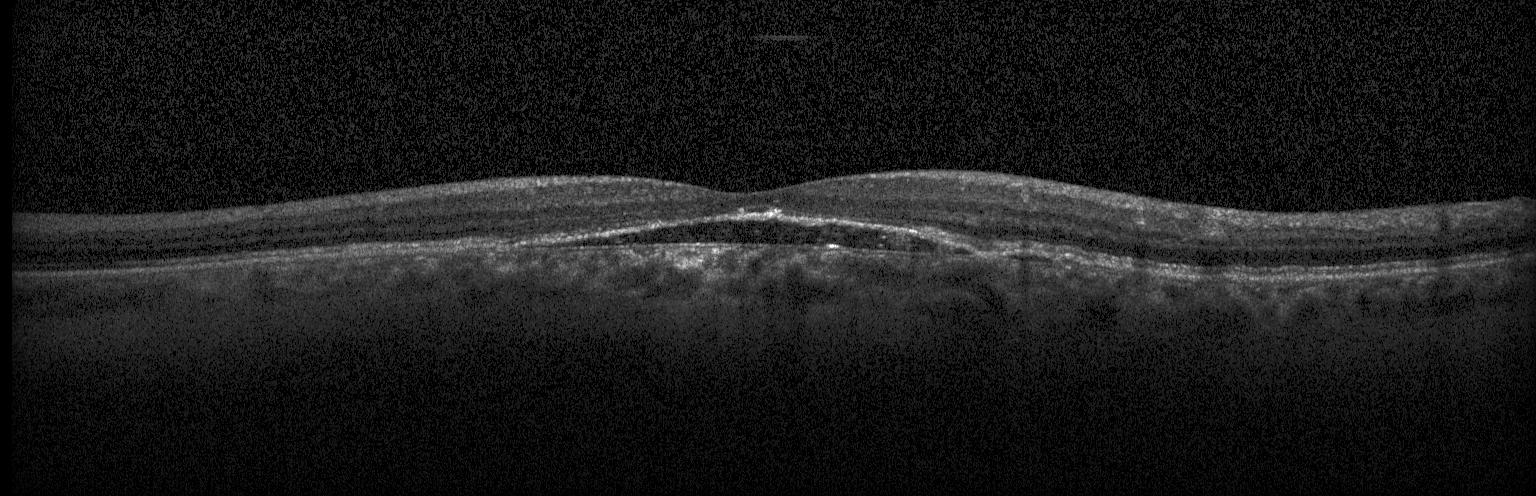

Spectral-domain optical coherence tomography; Heidelberg Spectralis; OCT line scan; through the macula. This B-scan demonstrates a choroidal neovascular membrane.